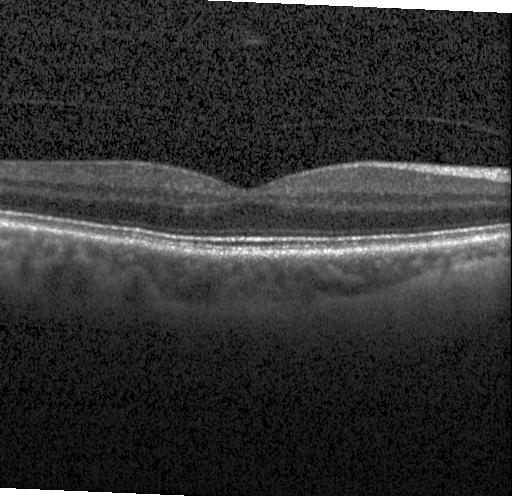

SD-OCT, Heidelberg Spectralis, optical coherence tomography B-scan. Finding: no CNV, DME, or drusen.